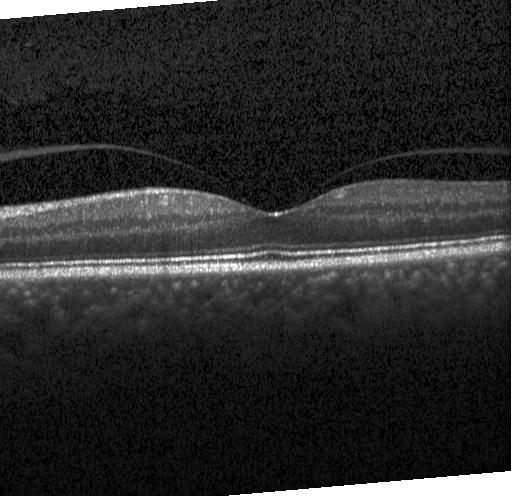

Spectral-domain optical coherence tomography. Optical coherence tomography scan. Through the macula. Acquired on a Heidelberg Spectralis. Diagnosis: no evidence of choroidal neovascularization, diabetic macular edema, or drusen.